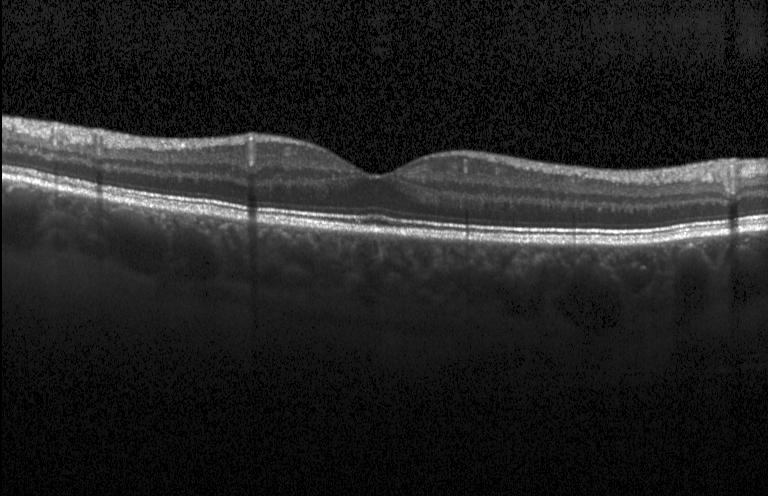
OCT line scan. Heidelberg Spectralis OCT system. Fovea-centered. SD-OCT.
Finding: neither CNV, DME, nor drusen.